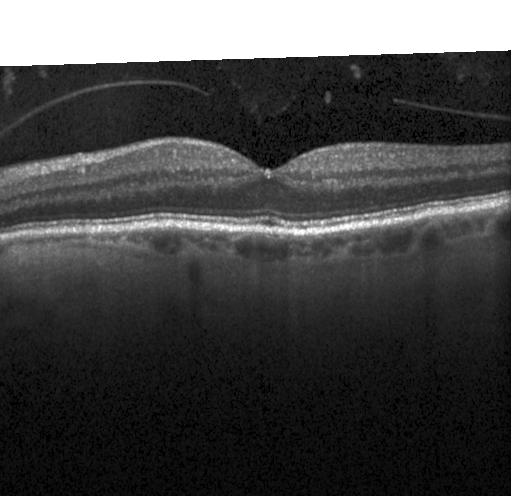 Retinal OCT cross-section
This B-scan demonstrates neither choroidal neovascularization, diabetic macular edema, nor drusen.